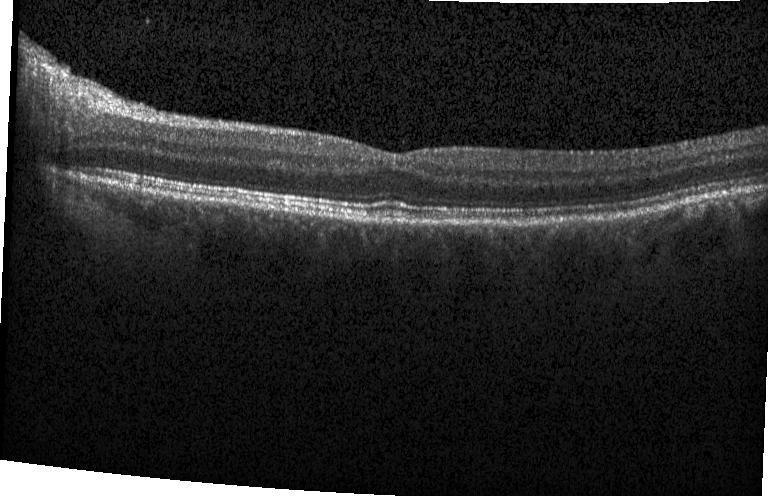 Instrument: Heidelberg Spectralis · optical coherence tomography B-scan — This B-scan demonstrates no CNV, DME, or drusen.